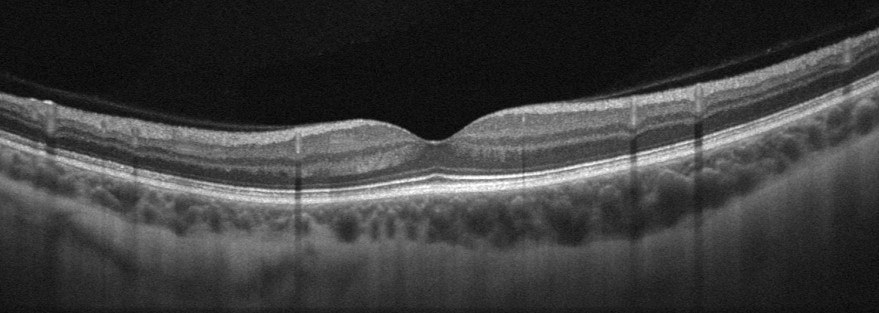

Optical coherence tomography B-scan. Through the macula
Diagnosis: no AMD, DME, ERM, RAO, RVO, or VID.